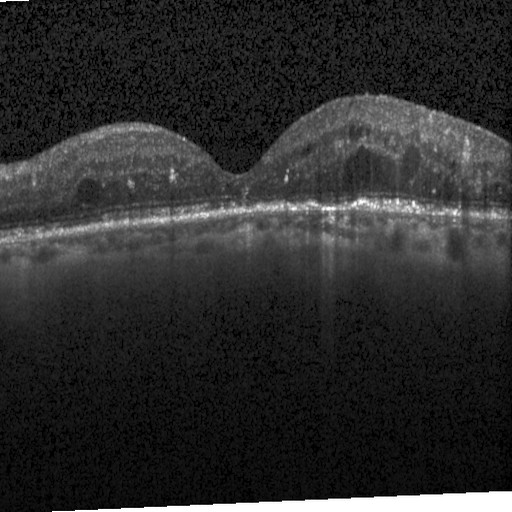 Heidelberg Spectralis · OCT line scan · horizontal scan through the fovea. Diabetic macular edema (DME).